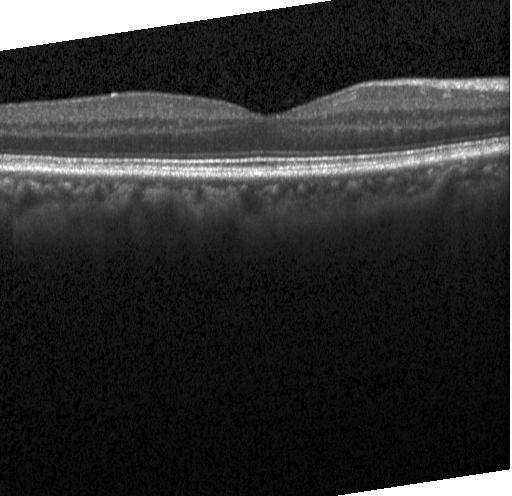 Finding: no evidence of choroidal neovascularization, diabetic macular edema, or drusen.